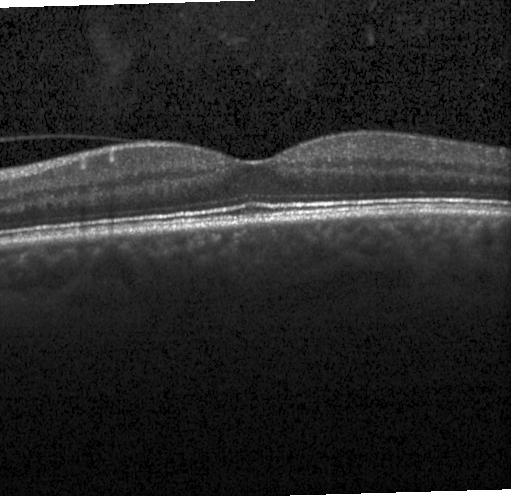 Instrument: Heidelberg Spectralis · OCT line scan. This B-scan demonstrates no CNV, no DME, and no drusen.